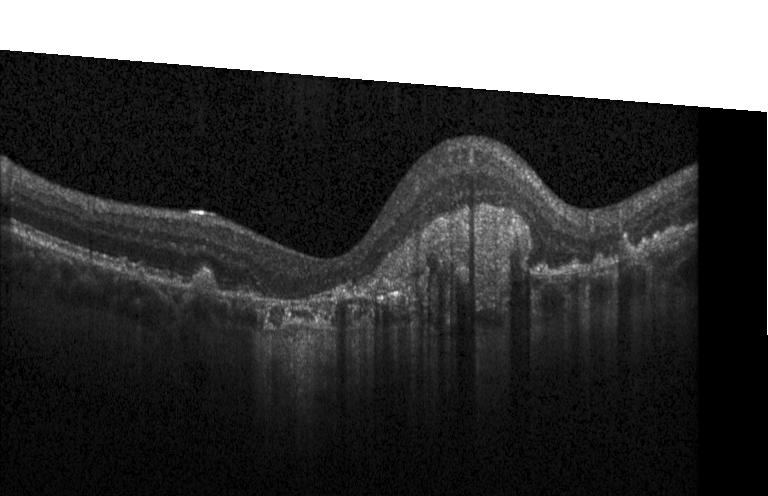

Diagnosis: choroidal neovascularization.